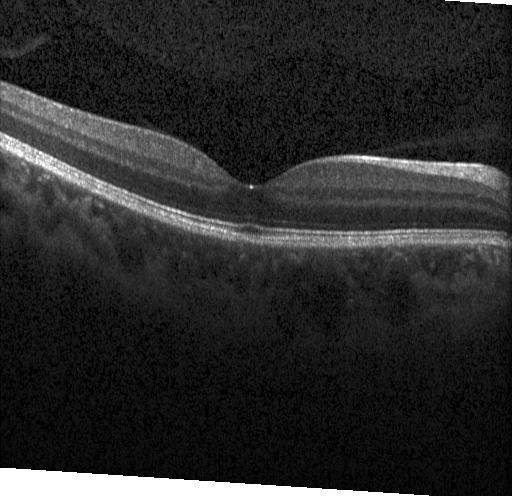 OCT finding: no choroidal neovascularization, no diabetic macular edema, and no drusen.